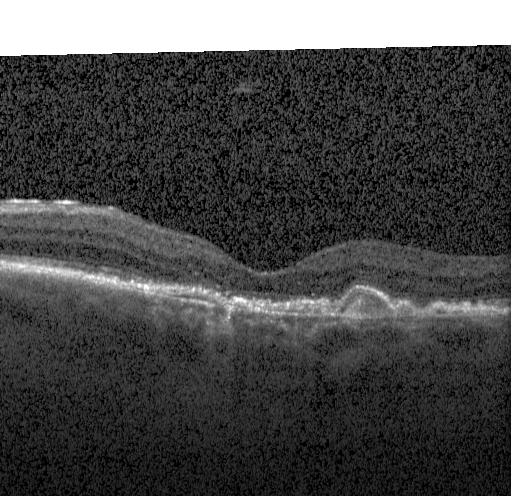
Impression: a choroidal neovascular membrane.